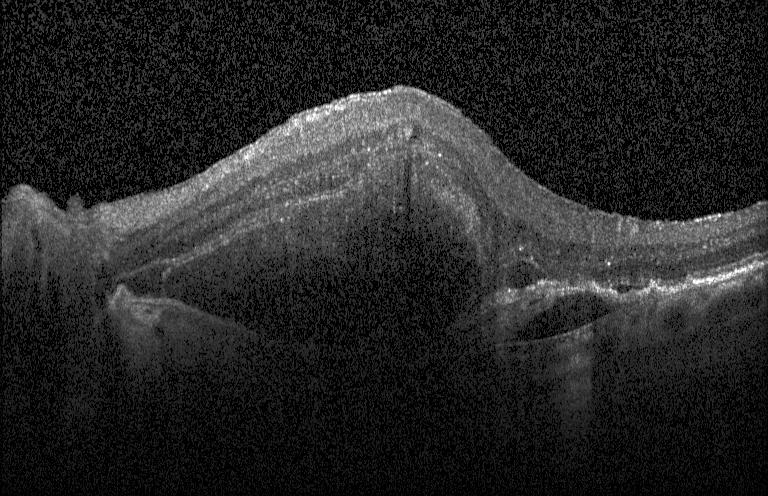 Optical coherence tomography scan
Impression: a choroidal neovascular membrane.